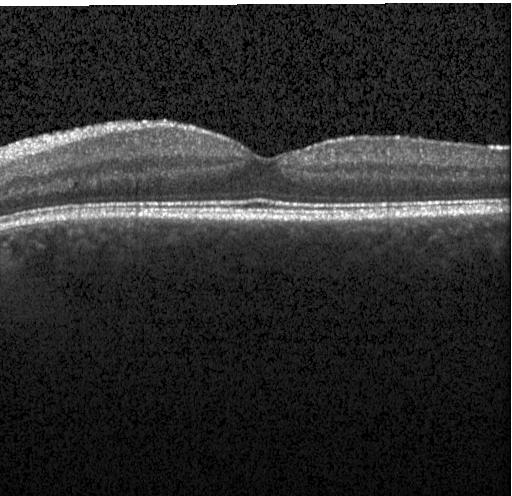

Macular OCT demonstrating neither choroidal neovascularization, diabetic macular edema, nor drusen.